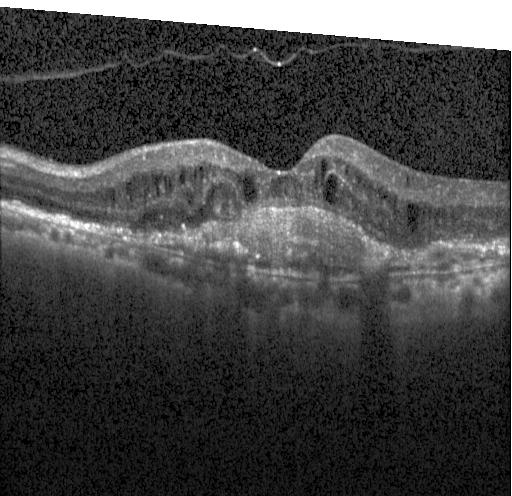 OCT scan showing a choroidal neovascular membrane.